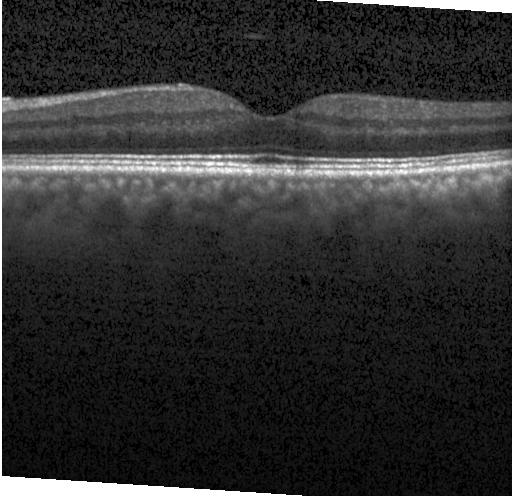

OCT B-scan showing no evidence of choroidal neovascularization, diabetic macular edema, or drusen.